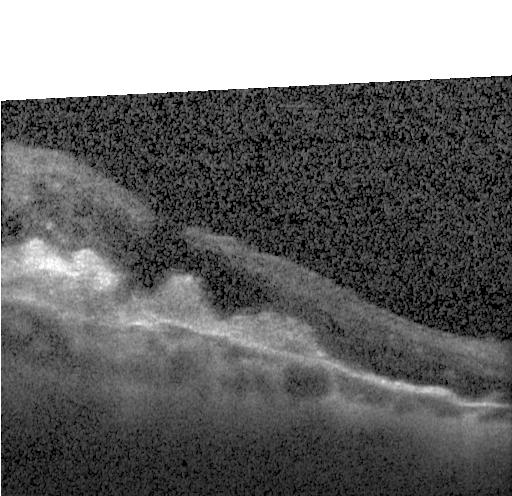

Spectral-domain optical coherence tomography. Centered on the fovea. Heidelberg Spectralis. Optical coherence tomography scan — Finding: CNV.